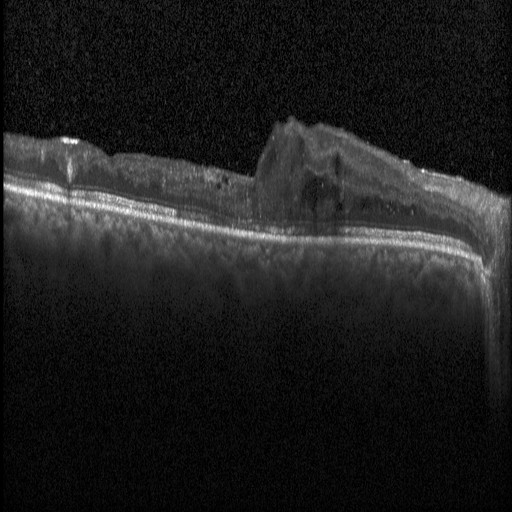

Diabetic macular edema (DME).